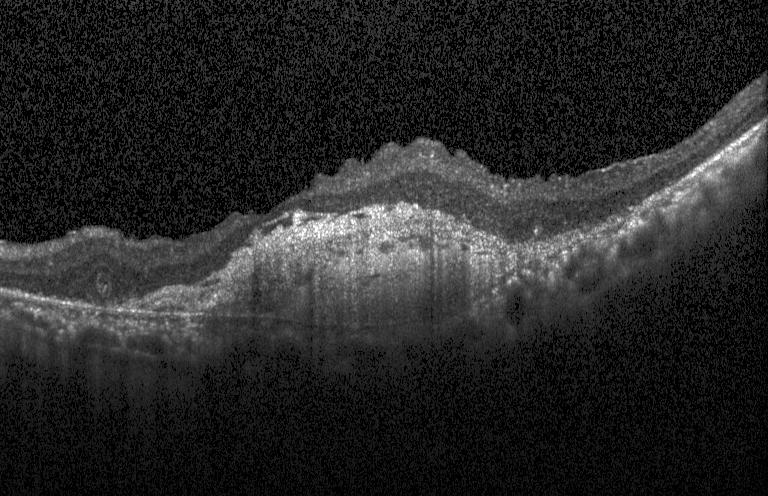 Macular OCT: CNV.